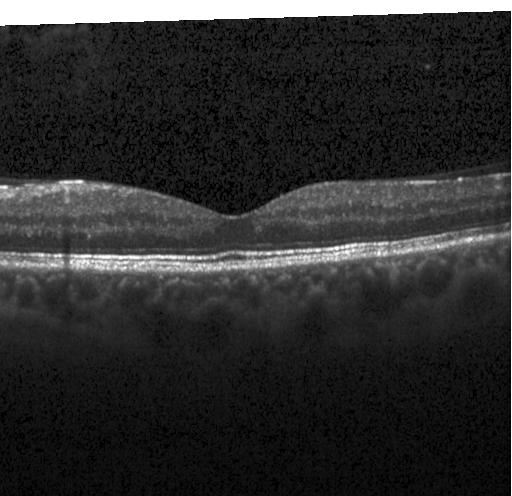

Fovea-centered. SD-OCT. Optical coherence tomography B-scan — Assessment: no CNV, no DME, and no drusen.